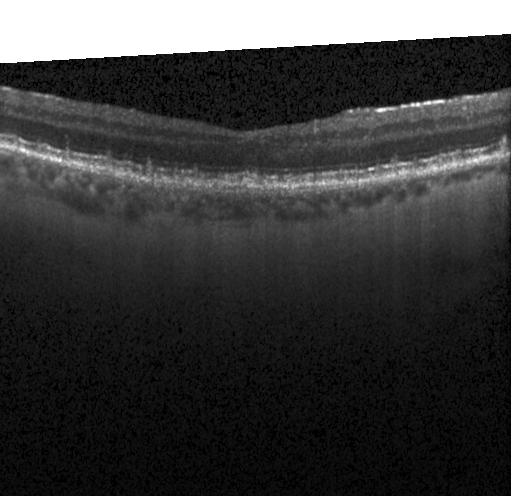 Impression: multiple drusen.